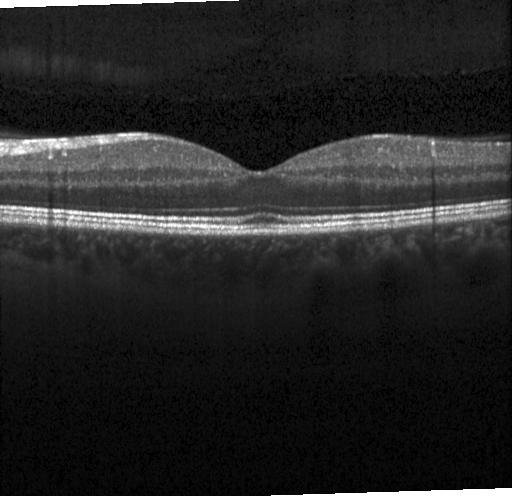 Centered on the fovea, Heidelberg Spectralis OCT system, retinal OCT B-scan, spectral-domain OCT
Finding: no evidence of CNV, DME, or drusen.